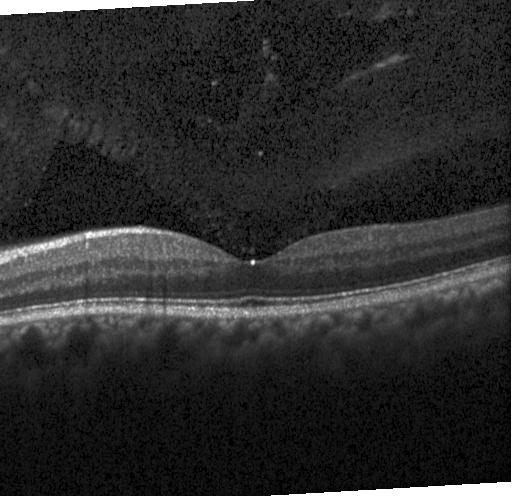

The scan shows no choroidal neovascularization, diabetic macular edema, or drusen.